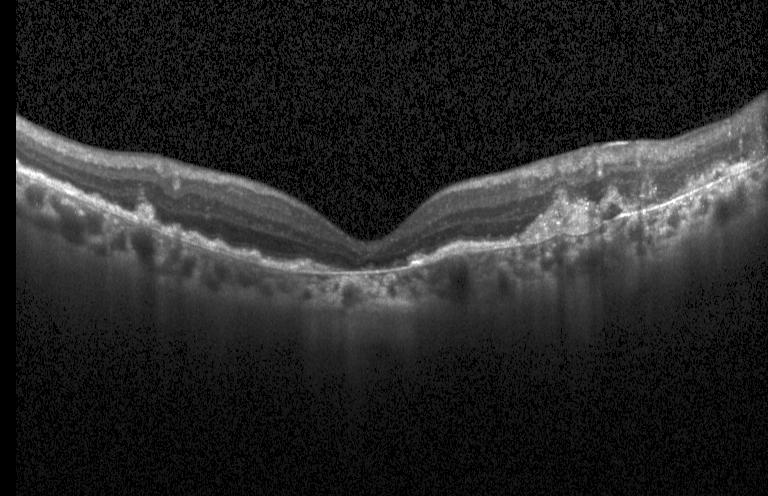

Diagnosis: a choroidal neovascular membrane.